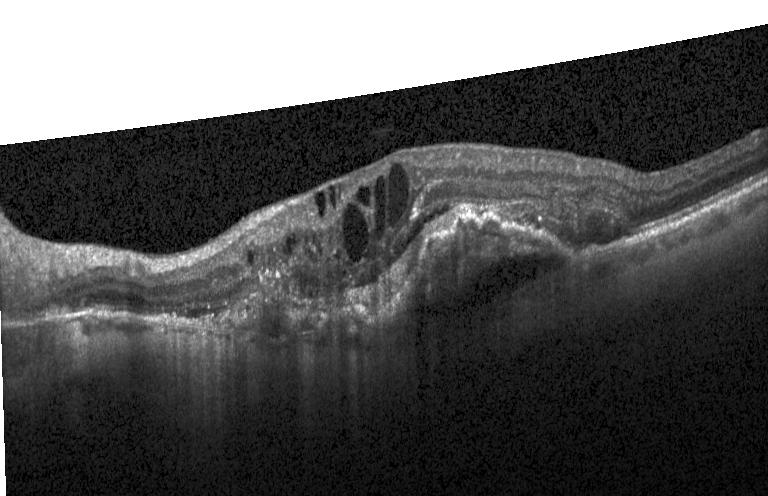

This B-scan demonstrates a choroidal neovascular membrane.